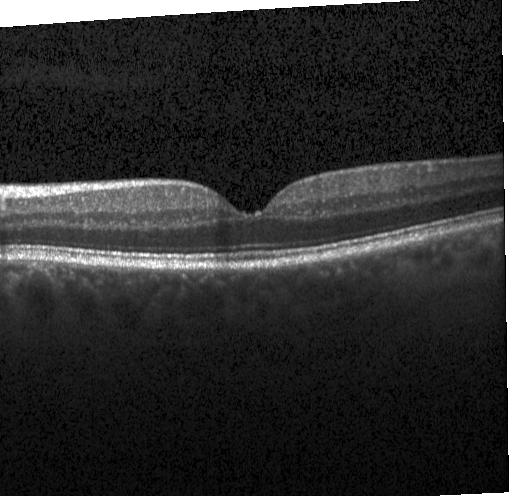

Spectral-domain OCT · fovea-centered · optical coherence tomography scan
Assessment: no evidence of CNV, DME, or drusen.